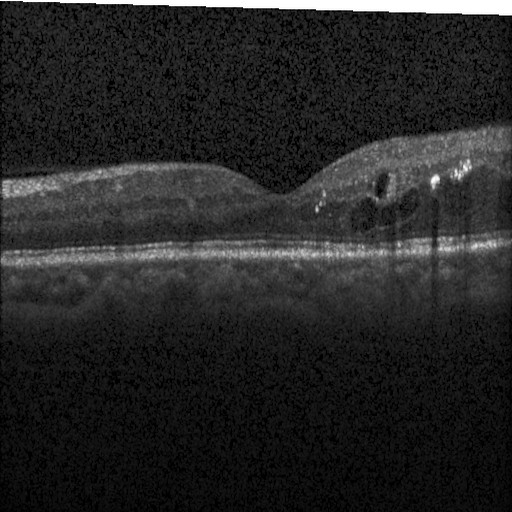

Heidelberg Spectralis. Optical coherence tomography scan
Diagnosis: diabetic macular edema (DME).